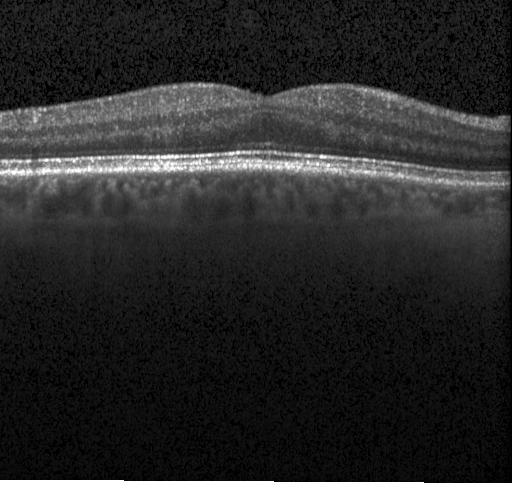 OCT line scan · Heidelberg Spectralis
Impression: no CNV, DME, or drusen.